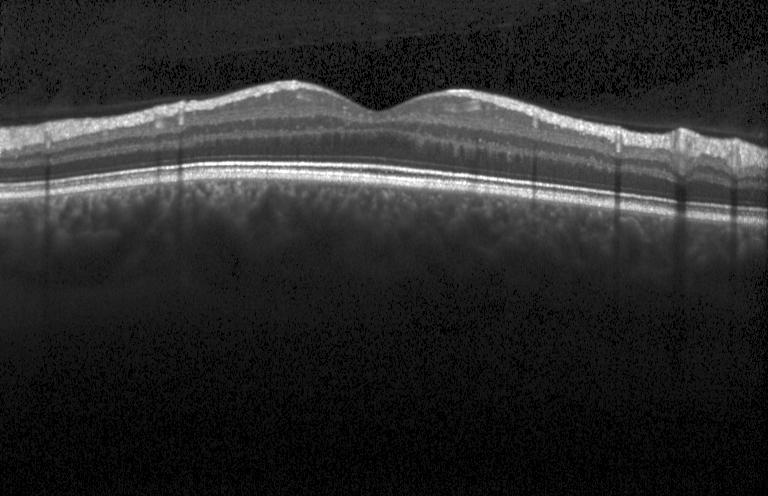

No choroidal neovascularization, diabetic macular edema, or drusen.